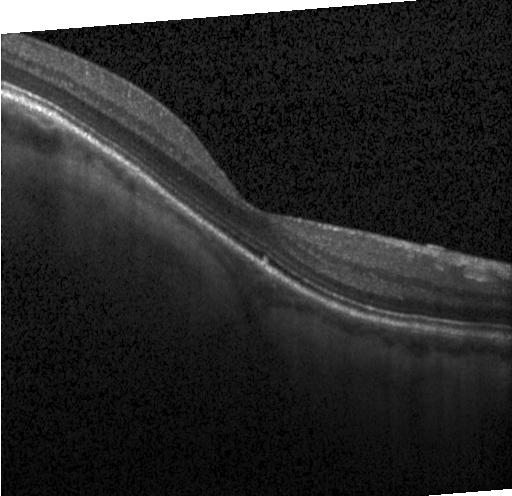
Macular OCT: neither choroidal neovascularization, diabetic macular edema, nor drusen.